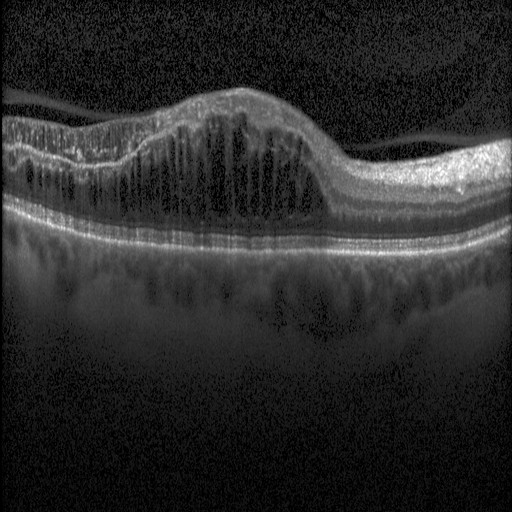
OCT B-scan · macular scan · SD-OCT
This B-scan demonstrates diabetic macular edema.